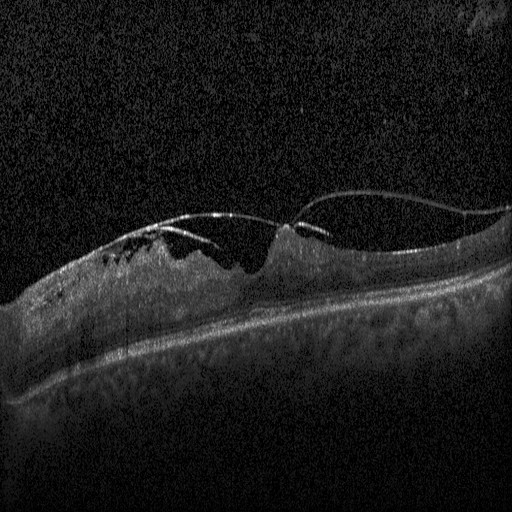
Instrument: Heidelberg Spectralis · SD-OCT · fovea-centered · retinal OCT B-scan
Assessment: DME.